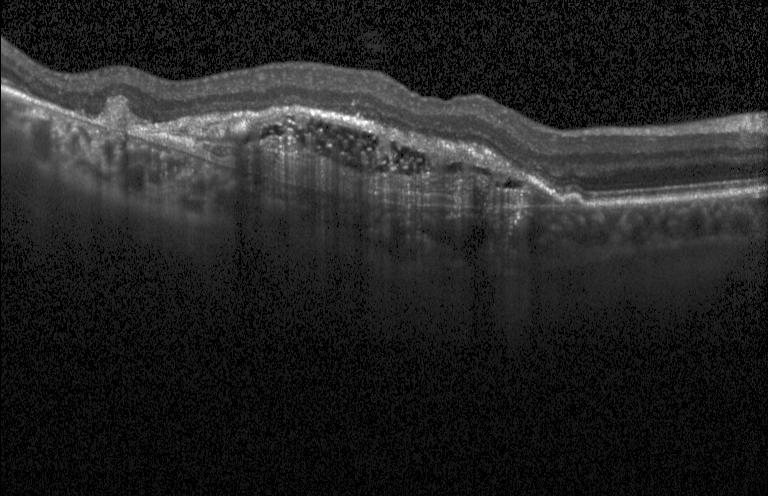 Spectral-domain OCT. Optical coherence tomography B-scan. Heidelberg Spectralis OCT system — Choroidal neovascularization (CNV).